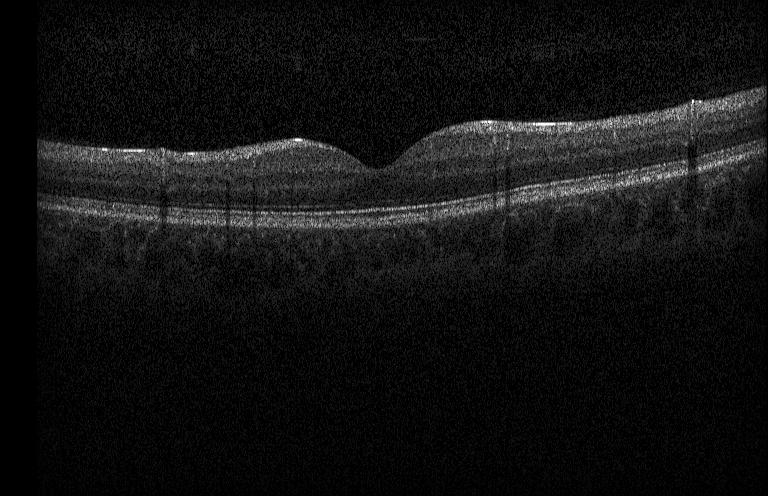

This B-scan demonstrates neither CNV, DME, nor drusen.